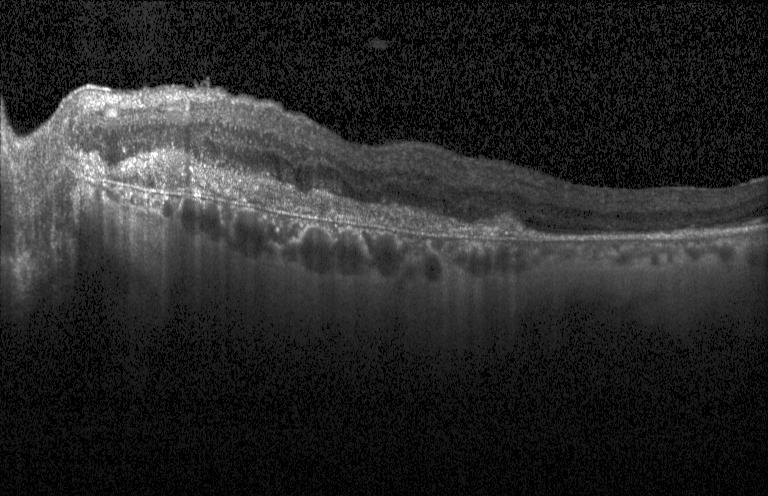

Optical coherence tomography scan
Finding: a choroidal neovascular membrane.